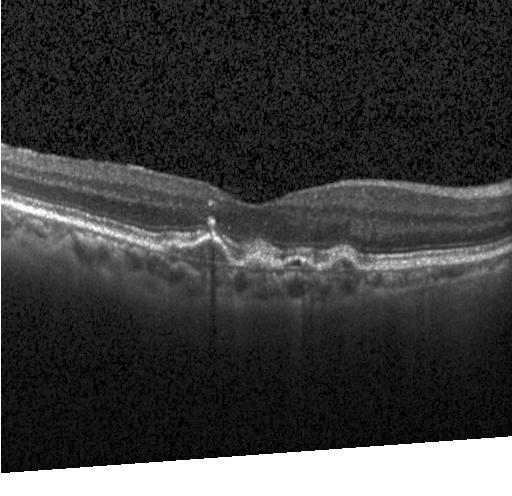
Spectral-domain OCT B-scan: a choroidal neovascular membrane.